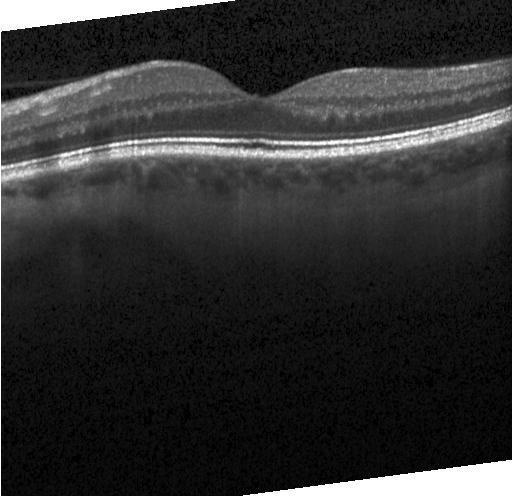 Fovea-centered · optical coherence tomography scan. Finding: neither CNV, DME, nor drusen.